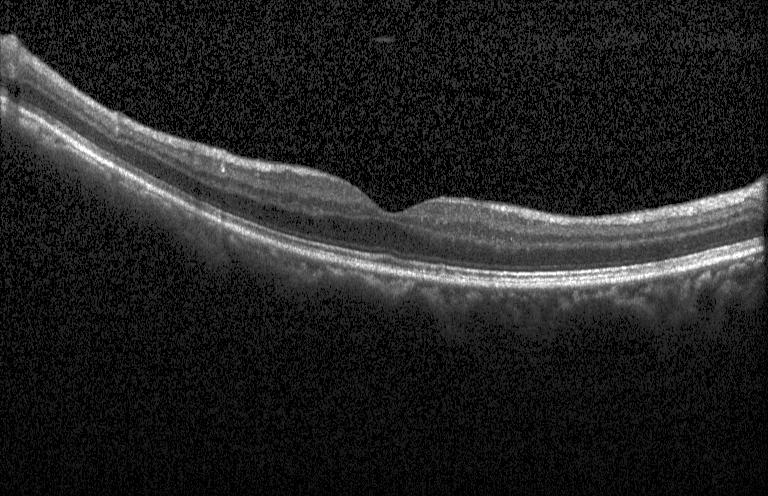 OCT line scan. Spectral-domain optical coherence tomography — Assessment: no evidence of choroidal neovascularization, diabetic macular edema, or drusen.